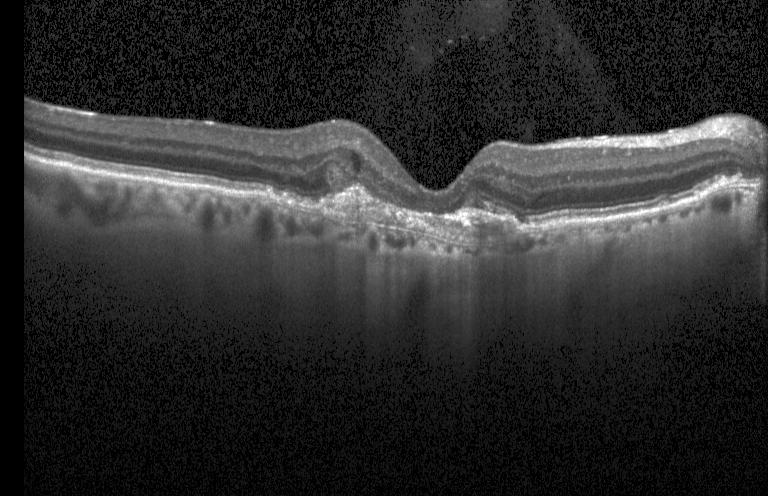 Retinal OCT B-scan, spectral-domain optical coherence tomography, acquired on a Heidelberg Spectralis.
A choroidal neovascular membrane.